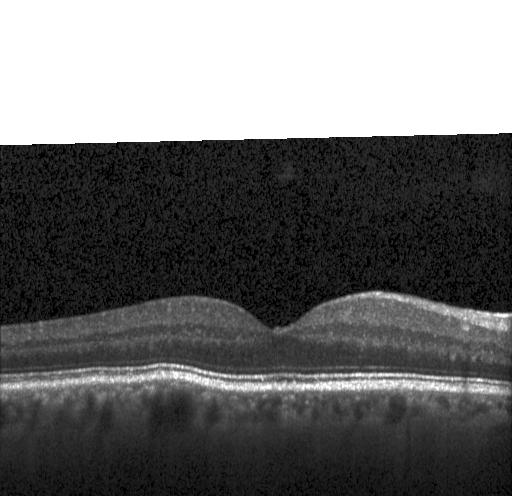
Retinal OCT B-scan · spectral-domain OCT · horizontal scan through the fovea · Heidelberg Spectralis
Impression: no evidence of choroidal neovascularization, diabetic macular edema, or drusen.